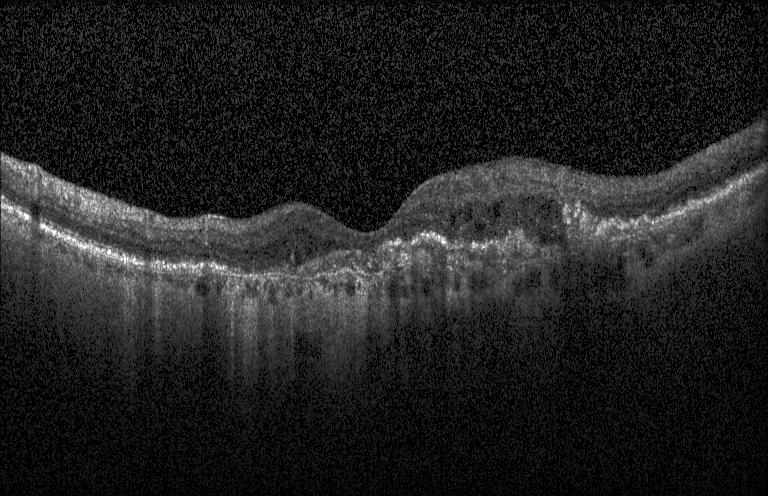 Through the macula. Acquired on a Heidelberg Spectralis. OCT B-scan. Spectral-domain OCT. Dx: choroidal neovascularization.